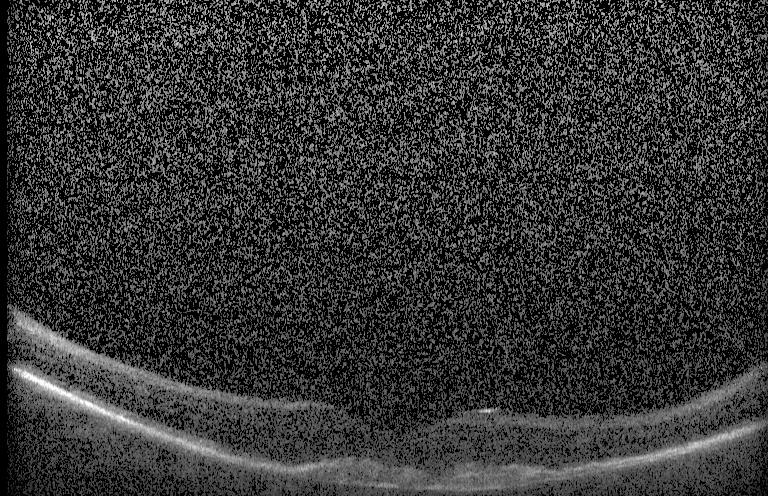
Retinal OCT B-scan, Heidelberg Spectralis. Impression: choroidal neovascularization (CNV).